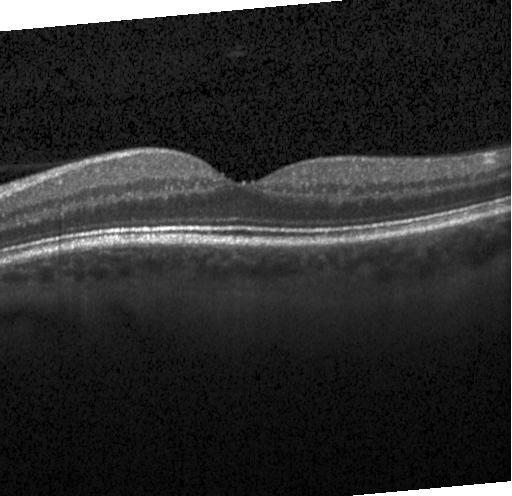
Diagnosis: neither choroidal neovascularization, diabetic macular edema, nor drusen.